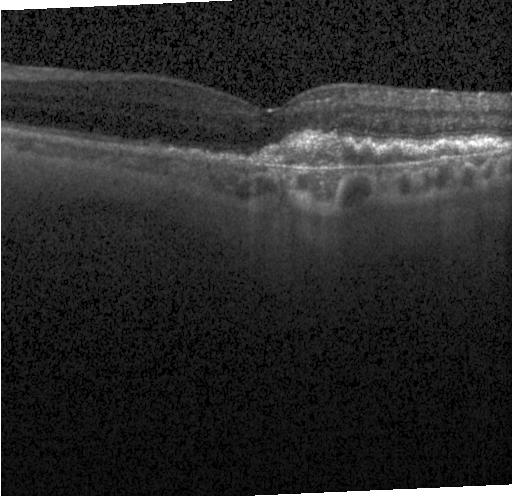

OCT B-scan showing CNV.